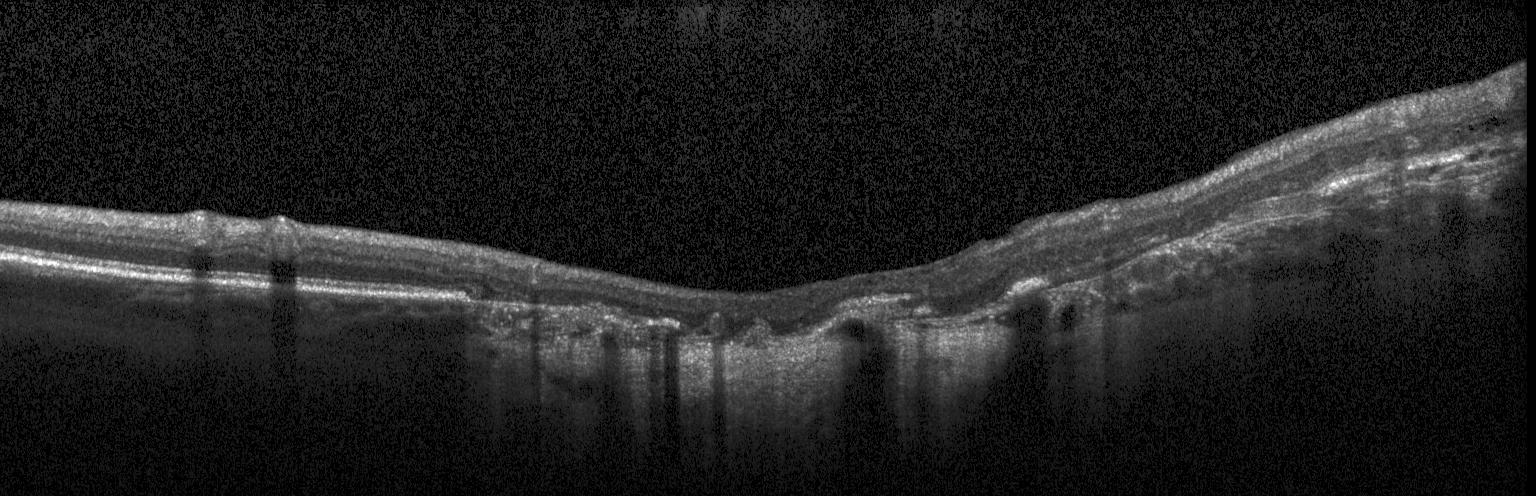
OCT line scan, through the macula, spectral-domain OCT. Dx: a choroidal neovascular membrane.